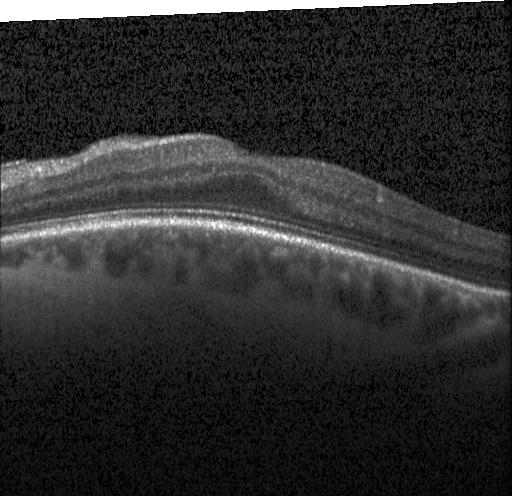

Dx: no evidence of choroidal neovascularization, diabetic macular edema, or drusen.